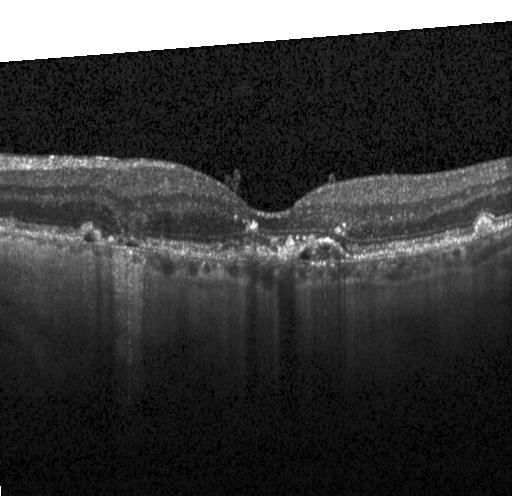 Horizontal scan through the fovea. Spectral-domain OCT. Optical coherence tomography scan — Diagnosis: choroidal neovascularization (CNV).